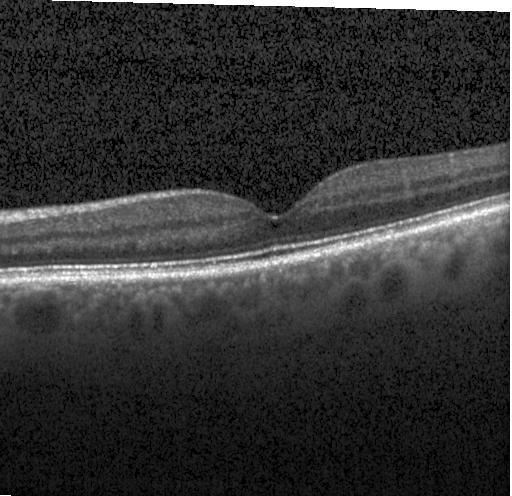 OCT B-scan · SD-OCT
Diagnosis: no CNV, no DME, and no drusen.